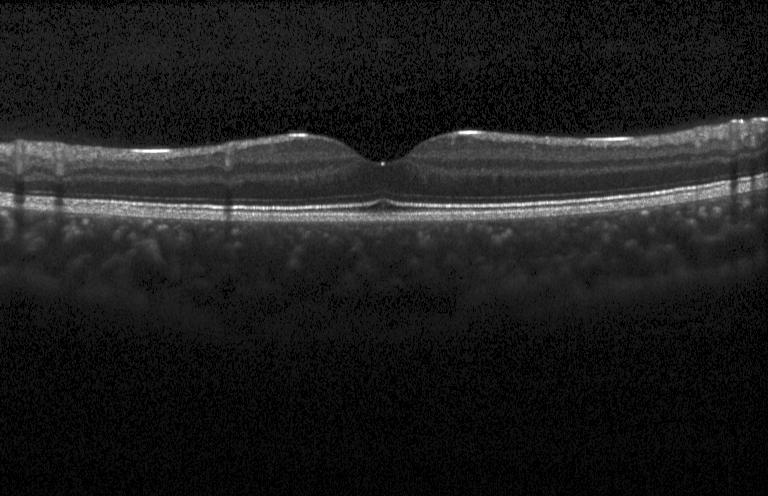
Macular OCT: no choroidal neovascularization, diabetic macular edema, or drusen.